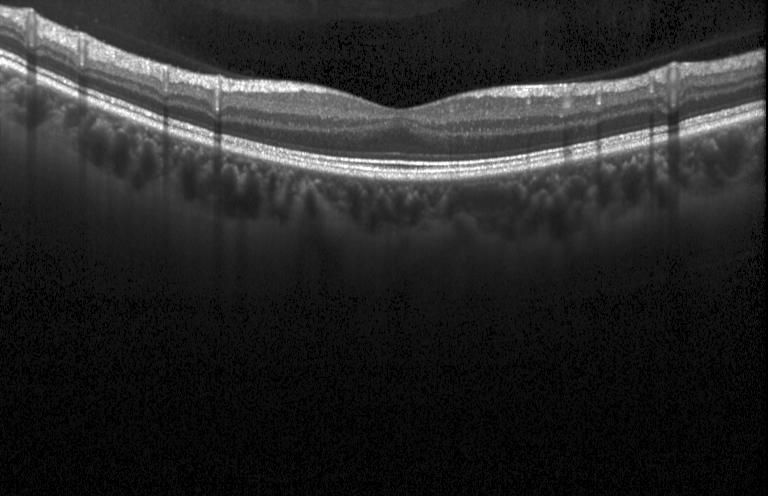

Heidelberg Spectralis, macular scan, optical coherence tomography scan, spectral-domain optical coherence tomography. Finding: no CNV, DME, or drusen.